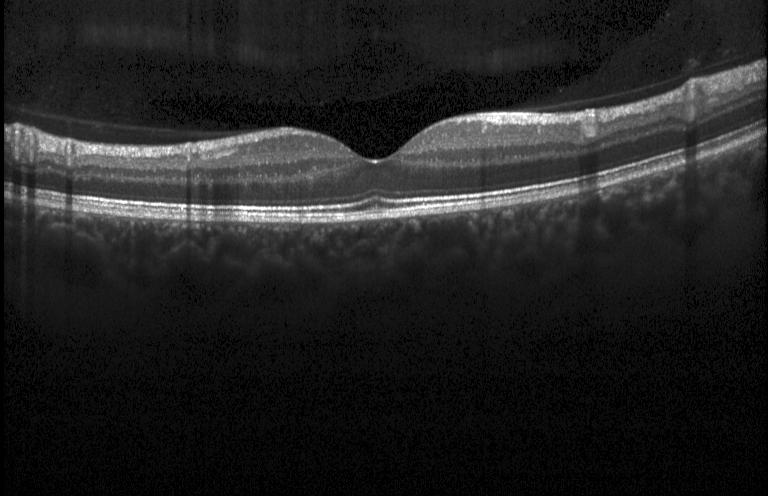

Horizontal scan through the fovea · Heidelberg Spectralis · SD-OCT · optical coherence tomography scan — The scan shows no choroidal neovascularization, diabetic macular edema, or drusen.